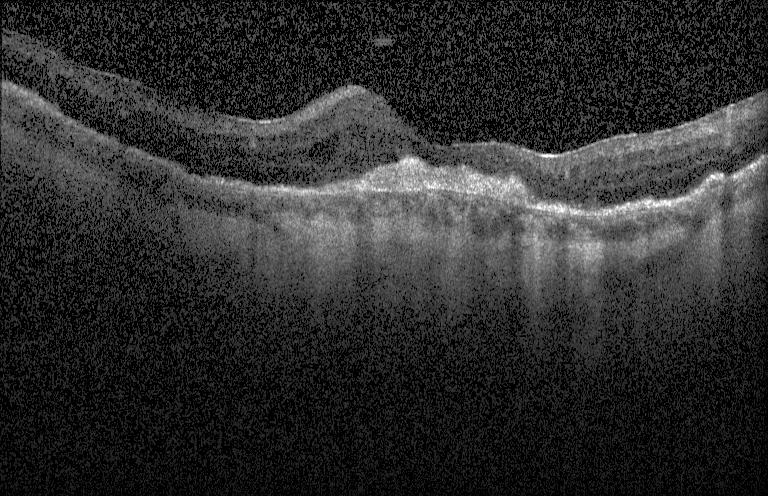
Assessment: CNV.